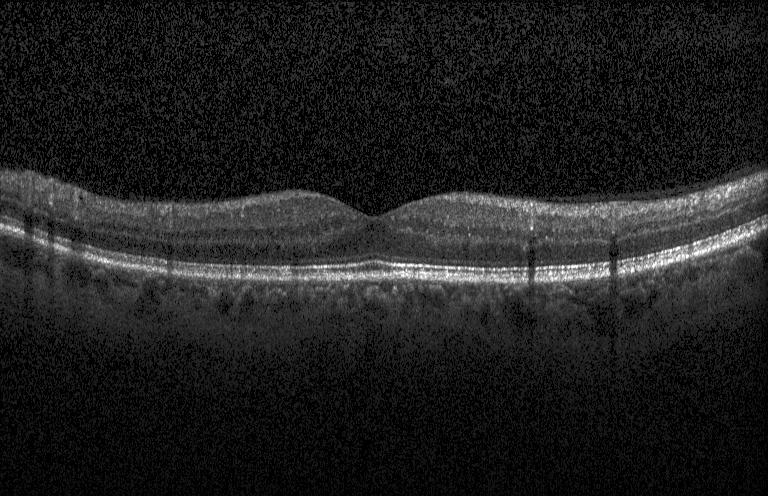 Macular OCT: no CNV, DME, or drusen.